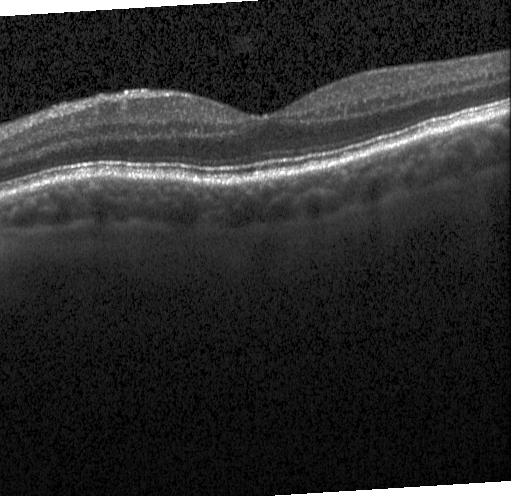

Horizontal scan through the fovea, optical coherence tomography scan, acquired on a Heidelberg Spectralis, spectral-domain optical coherence tomography
Assessment: no choroidal neovascularization, no diabetic macular edema, and no drusen.